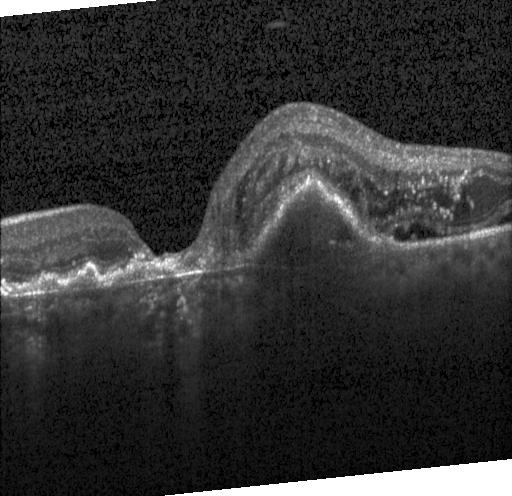
Diagnosis: CNV.